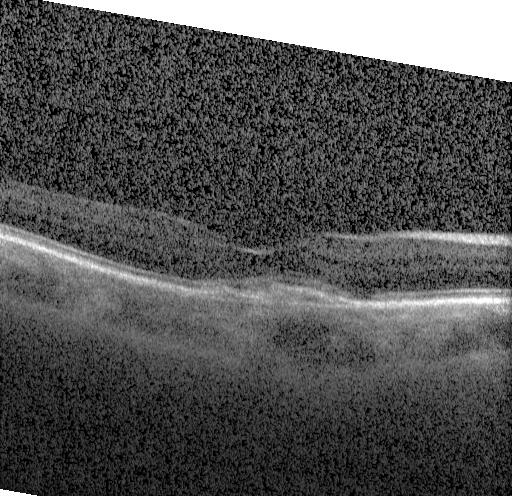

Impression: a choroidal neovascular membrane.